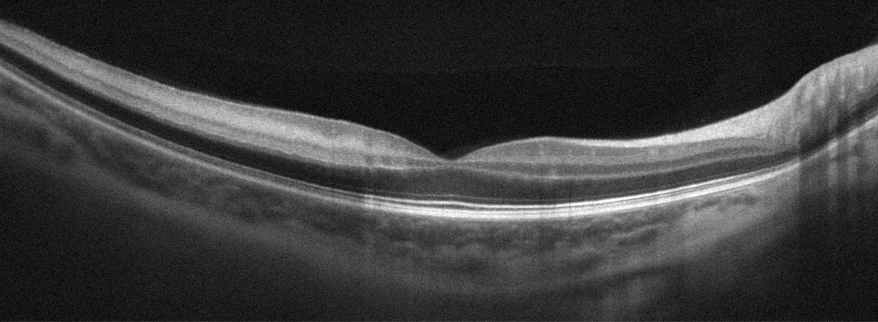 Retinal OCT cross-section — The scan shows retinal artery occlusion.